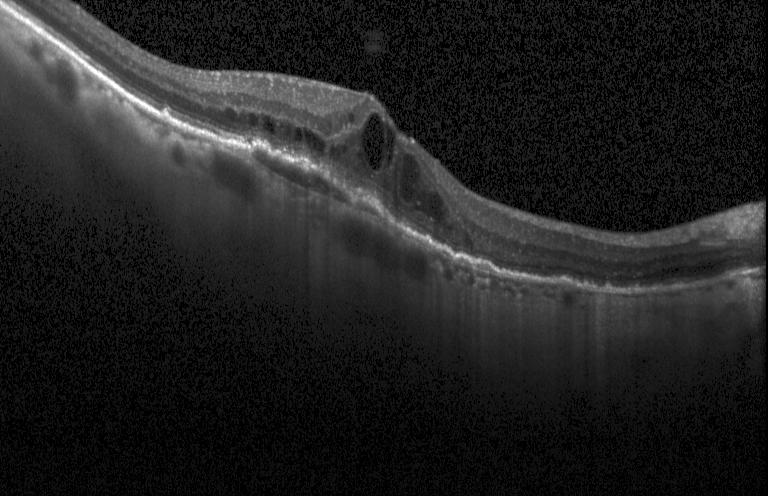

Fovea-centered, instrument: Heidelberg Spectralis, OCT B-scan. Dx: choroidal neovascularization (CNV).